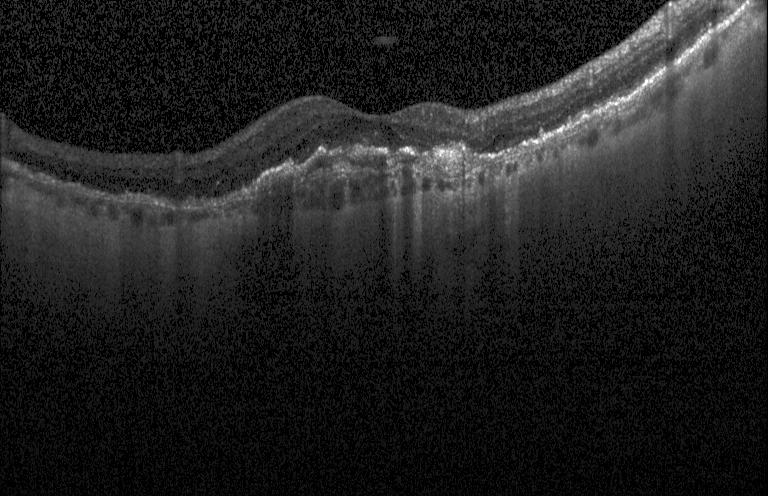 OCT scan showing choroidal neovascularization (CNV).